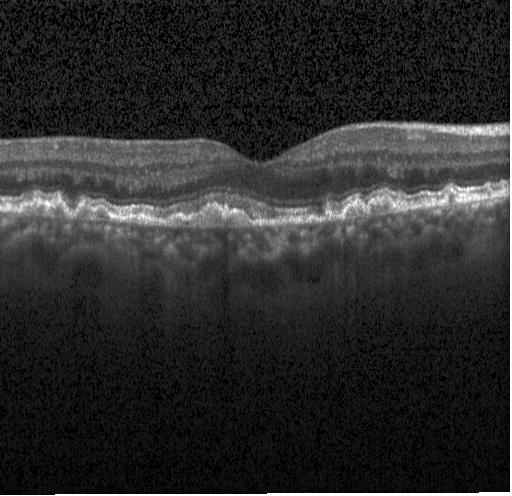 Through the macula, Heidelberg Spectralis, spectral-domain optical coherence tomography, OCT line scan.
This B-scan demonstrates sub-RPE drusenoid deposits.